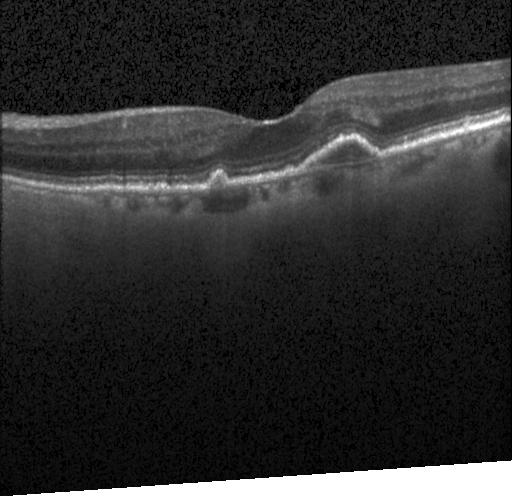
Retinal OCT cross-section showing a choroidal neovascular membrane.